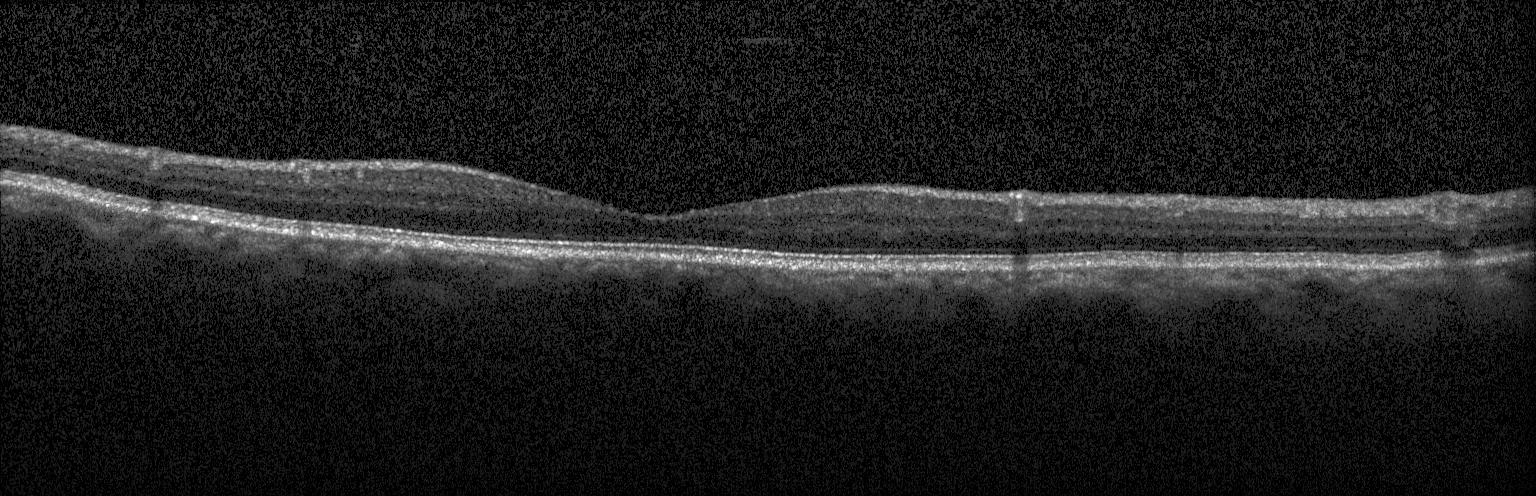 Diagnosis: no evidence of choroidal neovascularization, diabetic macular edema, or drusen.